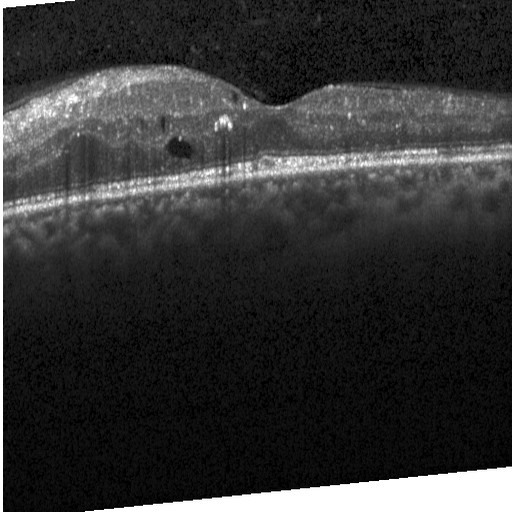 Instrument: Heidelberg Spectralis; spectral-domain optical coherence tomography; optical coherence tomography B-scan; horizontal scan through the fovea — Impression: DME.